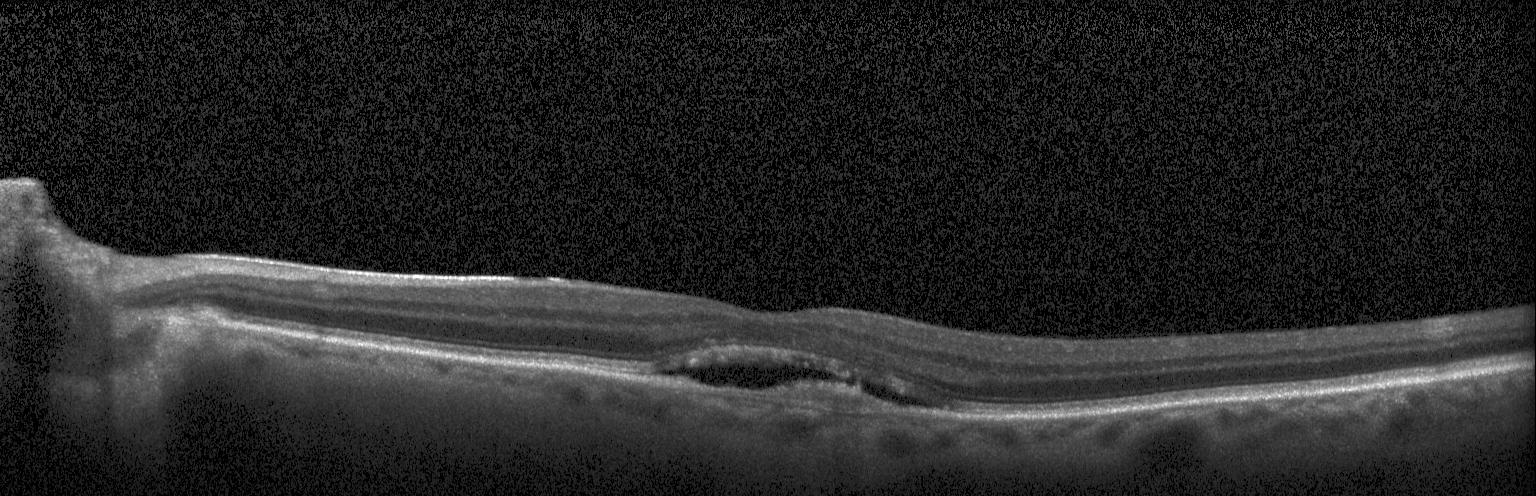

Diagnosis: a choroidal neovascular membrane.